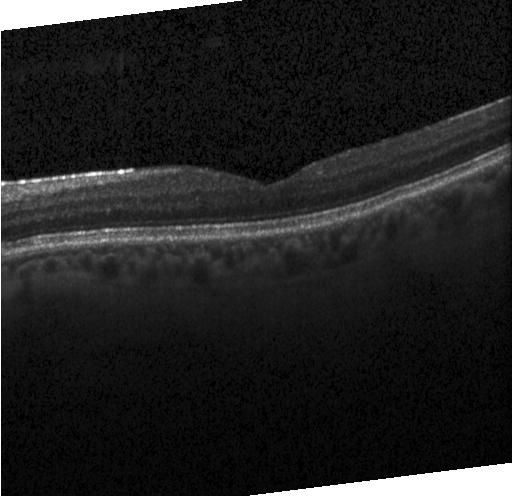

Retinal OCT cross-section, through the macula. Diagnosis: no CNV, no DME, and no drusen.